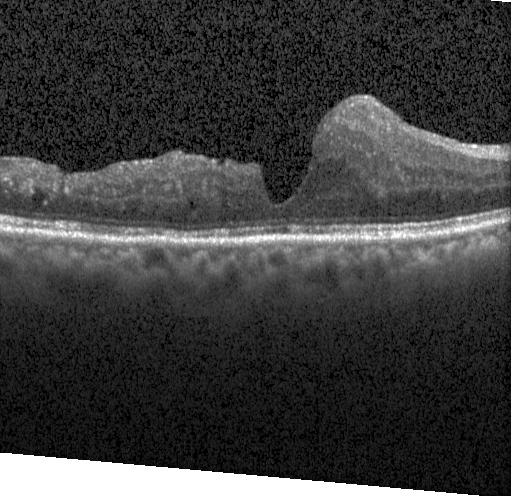 Macular scan; OCT line scan. Finding: diabetic macular edema.